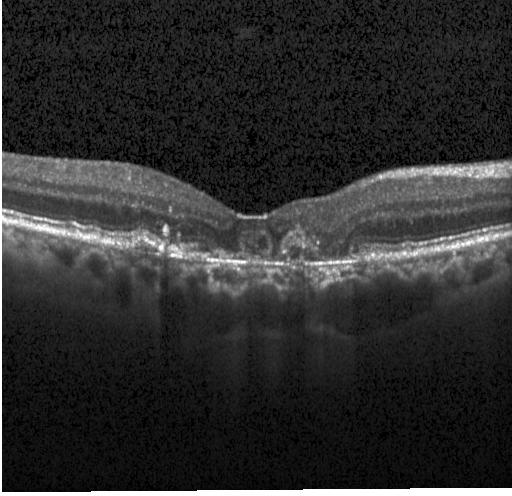

Retinal OCT cross-section. Spectral-domain optical coherence tomography.
Dx: choroidal neovascularization.